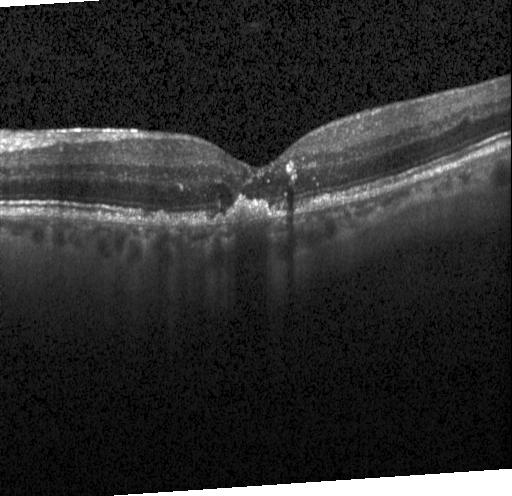
Retinal OCT B-scan; horizontal scan through the fovea.
Macular OCT: choroidal neovascularization.